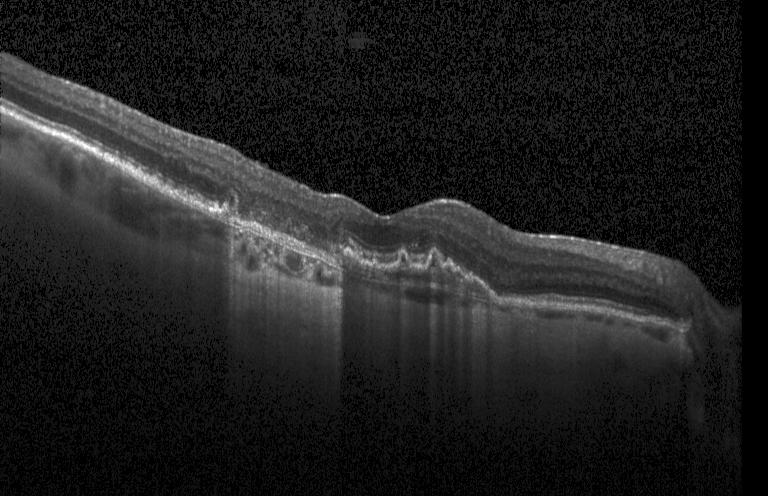 Diagnosis: CNV.